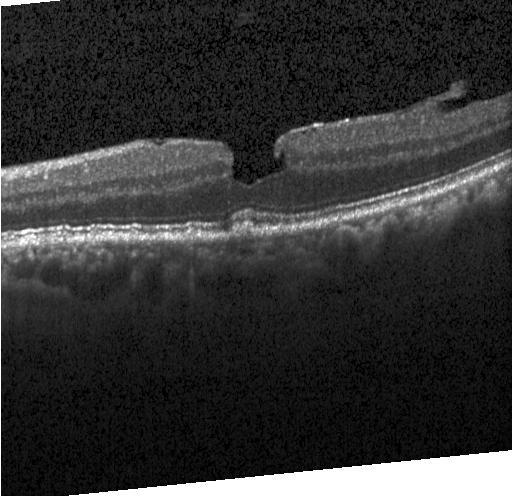

The scan shows drusen.